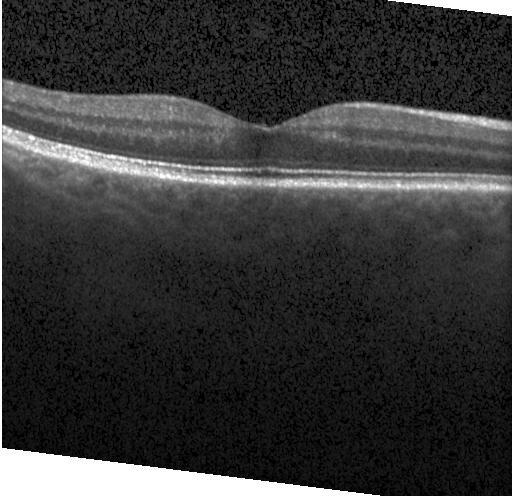 Retinal OCT cross-section; spectral-domain optical coherence tomography; Heidelberg Spectralis; horizontal scan through the fovea. The scan shows no choroidal neovascularization, diabetic macular edema, or drusen.